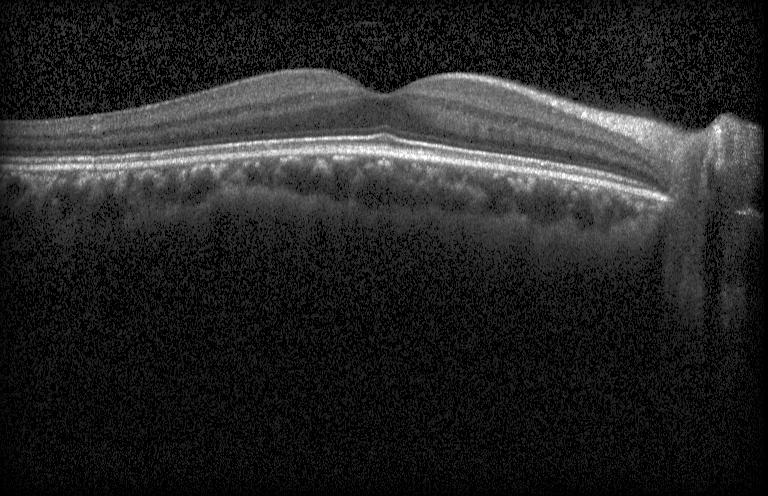 Instrument: Heidelberg Spectralis; retinal OCT B-scan; fovea-centered. Finding: no choroidal neovascularization, no diabetic macular edema, and no drusen.